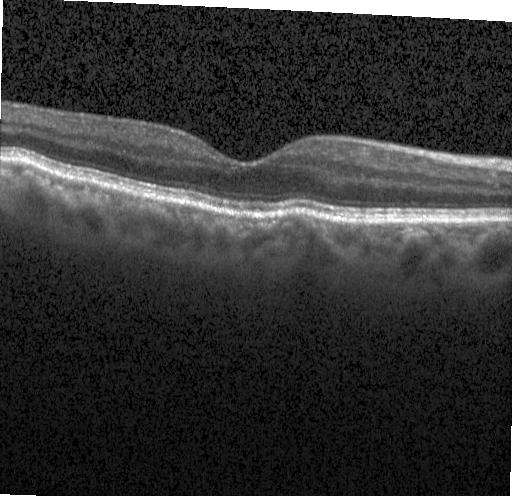 Spectral-domain optical coherence tomography, centered on the fovea, OCT line scan. Impression: no evidence of choroidal neovascularization, diabetic macular edema, or drusen.